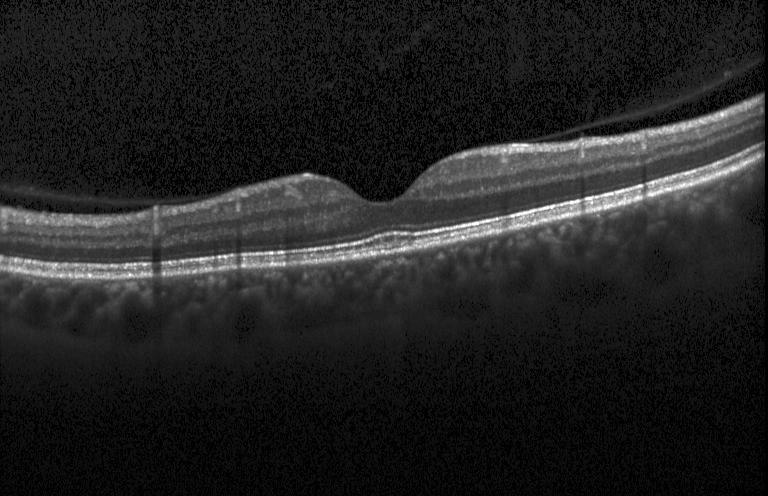
Finding: no choroidal neovascularization, diabetic macular edema, or drusen.